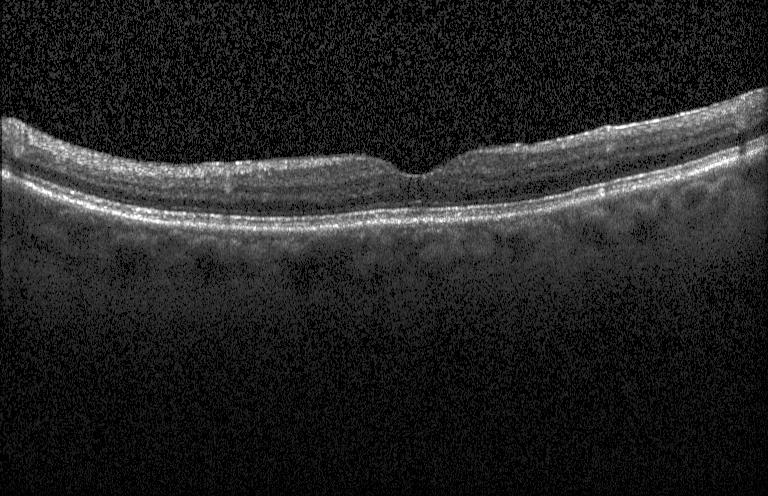 Retinal OCT B-scan; Heidelberg Spectralis; SD-OCT; macular scan — Impression: no choroidal neovascularization, no diabetic macular edema, and no drusen.